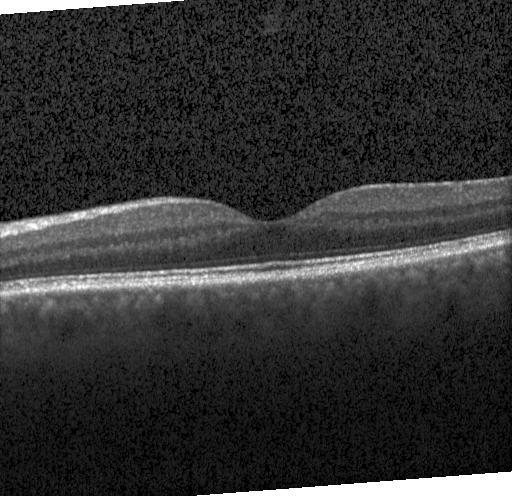

Retinal OCT B-scan.
Finding: no CNV, DME, or drusen.